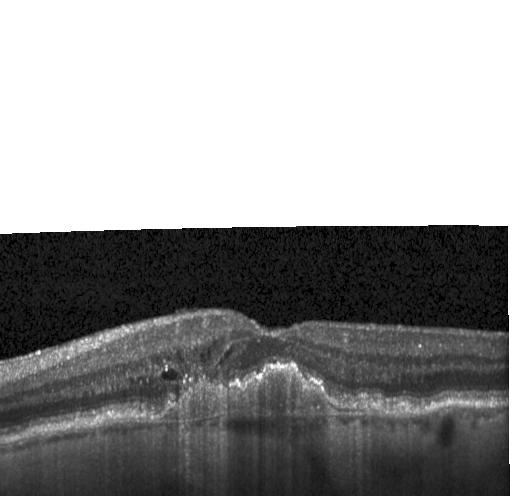 SD-OCT. OCT line scan. Fovea-centered — Assessment: a choroidal neovascular membrane.